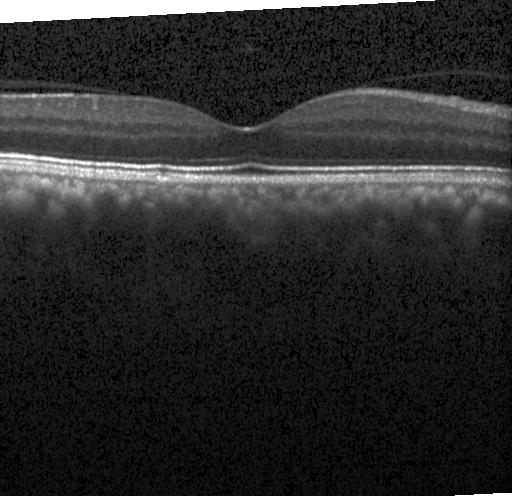 Spectral-domain OCT; OCT line scan; Heidelberg Spectralis OCT system — Finding: no choroidal neovascularization, diabetic macular edema, or drusen.